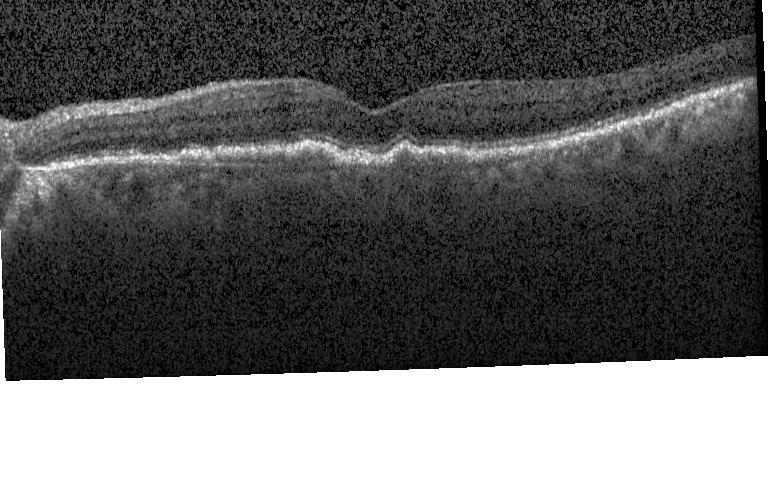
This B-scan demonstrates choroidal neovascularization.